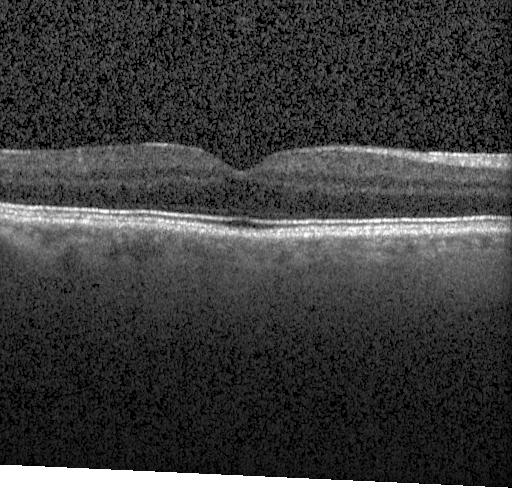

Retinal OCT B-scan. Horizontal scan through the fovea. Heidelberg Spectralis OCT system. Spectral-domain OCT
Impression: no choroidal neovascularization, no diabetic macular edema, and no drusen.